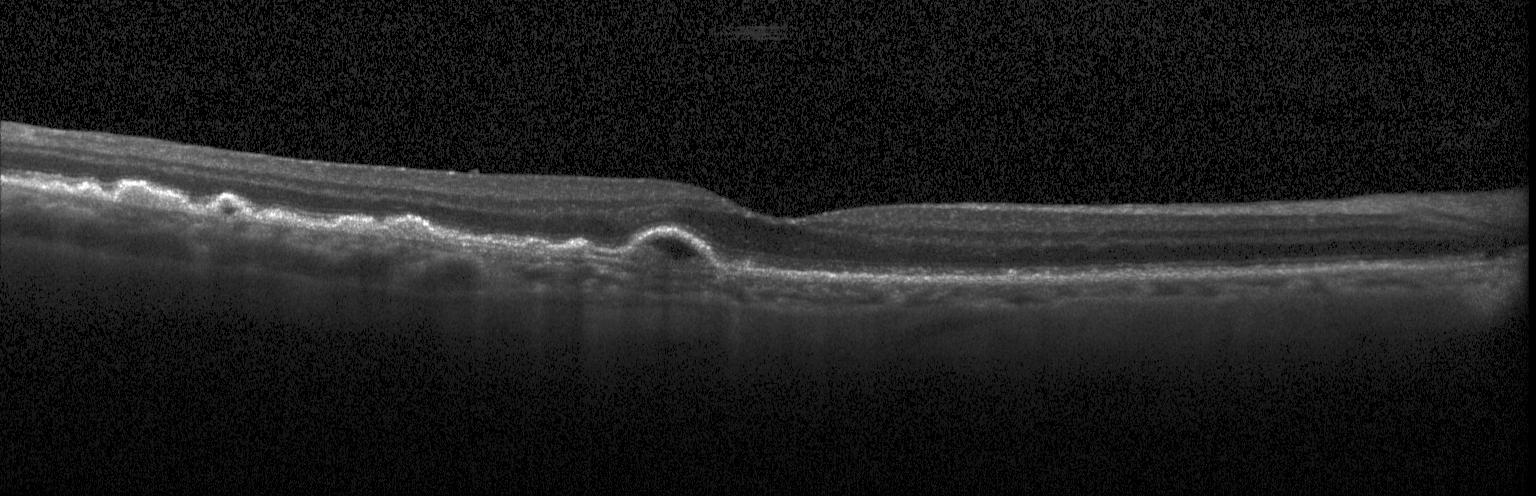 SD-OCT. Retinal OCT cross-section.
Impression: sub-RPE drusenoid deposits.